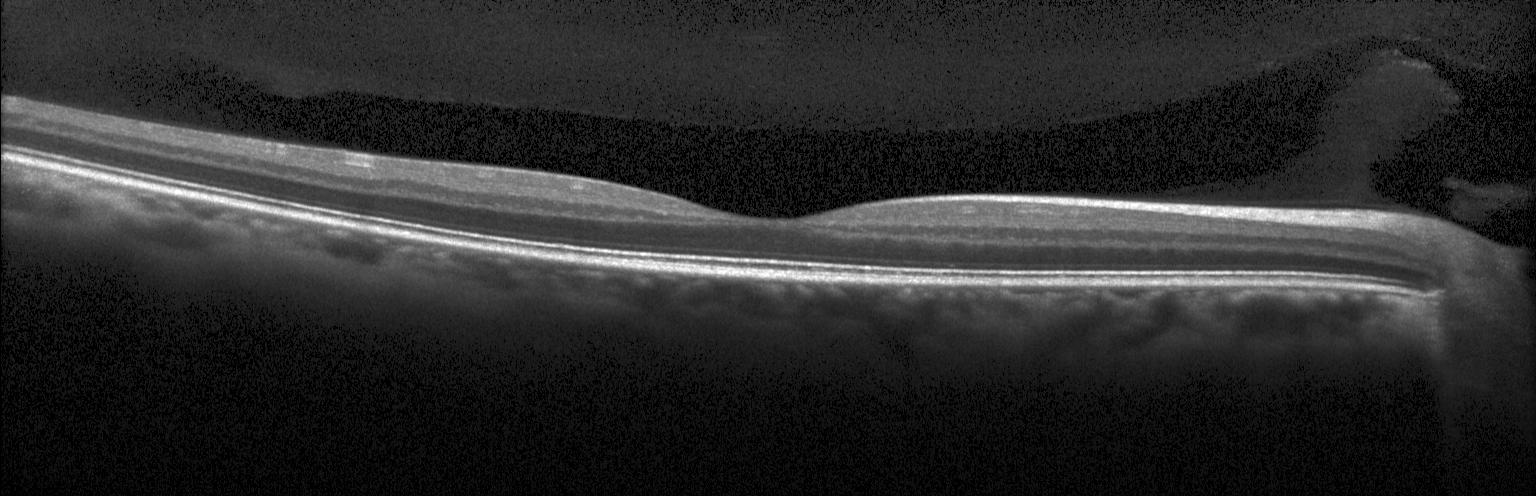

OCT B-scan. Macular OCT: neither choroidal neovascularization, diabetic macular edema, nor drusen.